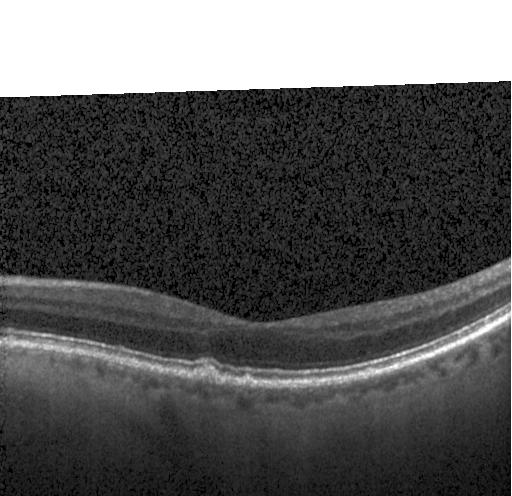
Spectral-domain OCT B-scan: sub-RPE drusenoid deposits.